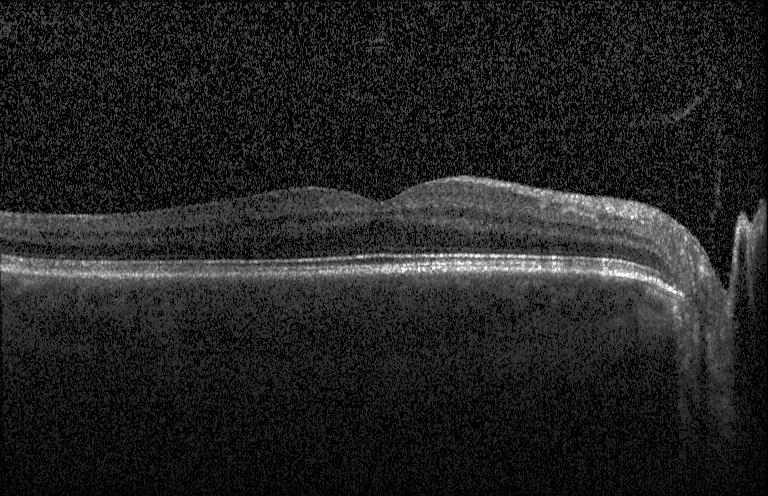 Optical coherence tomography scan. No evidence of choroidal neovascularization, diabetic macular edema, or drusen.